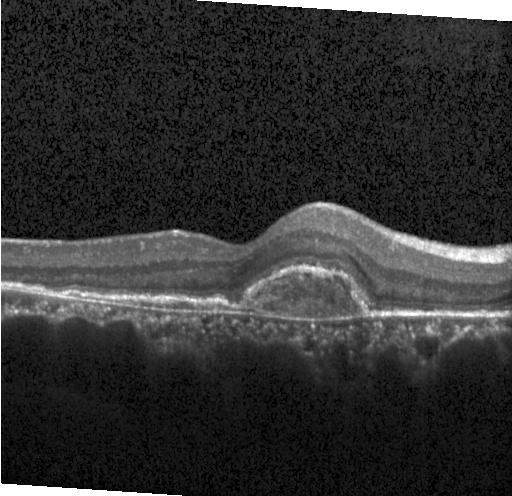

Finding: a choroidal neovascular membrane.